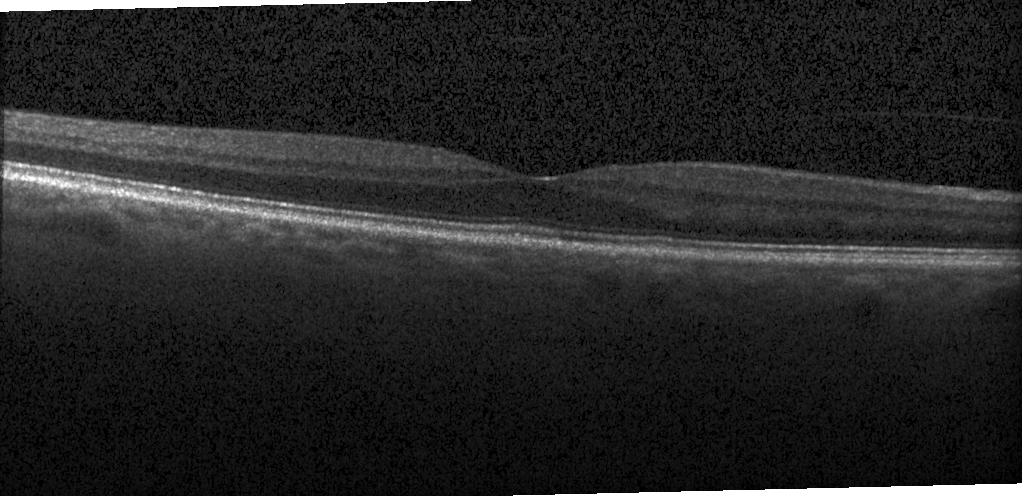

SD-OCT, retinal OCT cross-section, macular scan — Finding: no evidence of choroidal neovascularization, diabetic macular edema, or drusen.